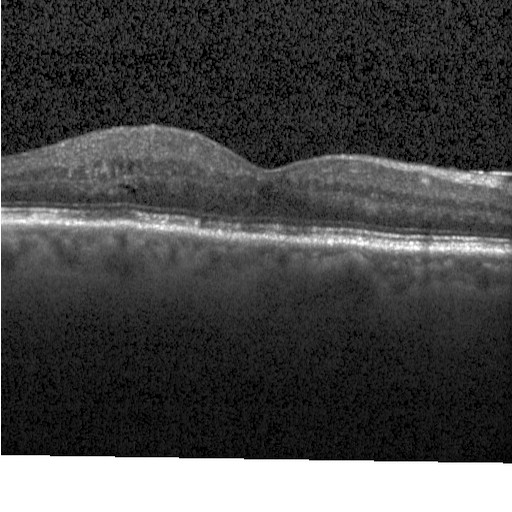 SD-OCT, optical coherence tomography scan, Heidelberg Spectralis OCT system, horizontal scan through the fovea — Diagnosis: diabetic macular edema (DME).